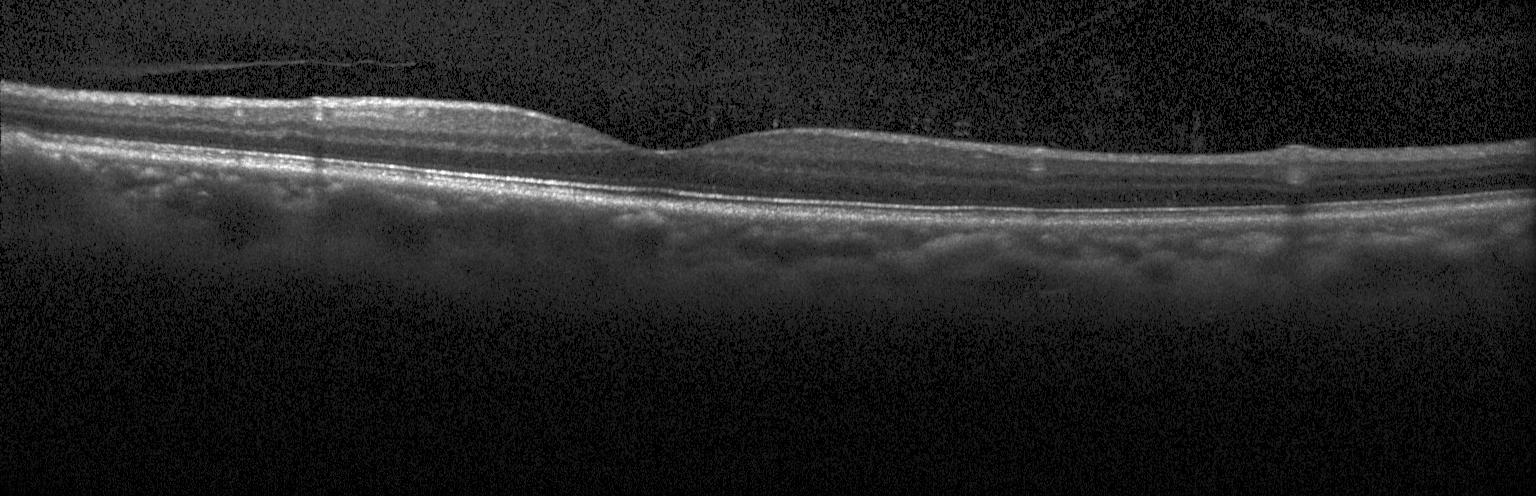
Macular OCT demonstrating no choroidal neovascularization, diabetic macular edema, or drusen.